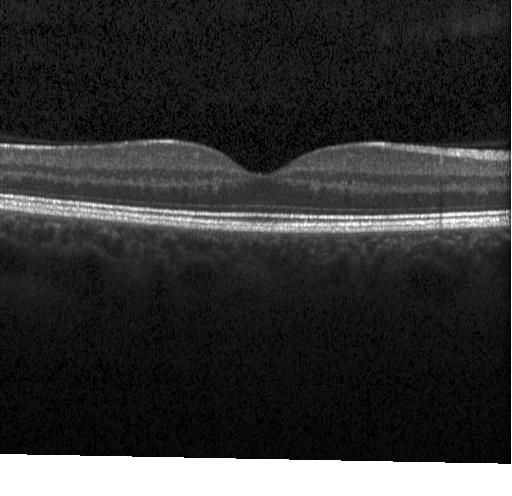 Through the macula; spectral-domain optical coherence tomography; instrument: Heidelberg Spectralis; optical coherence tomography scan
Assessment: no choroidal neovascularization, no diabetic macular edema, and no drusen.